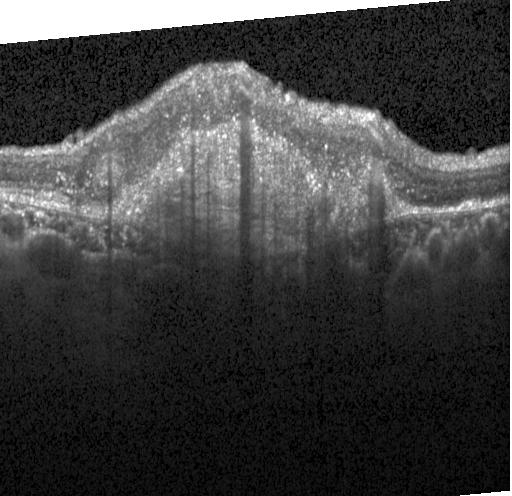
Impression: CNV.